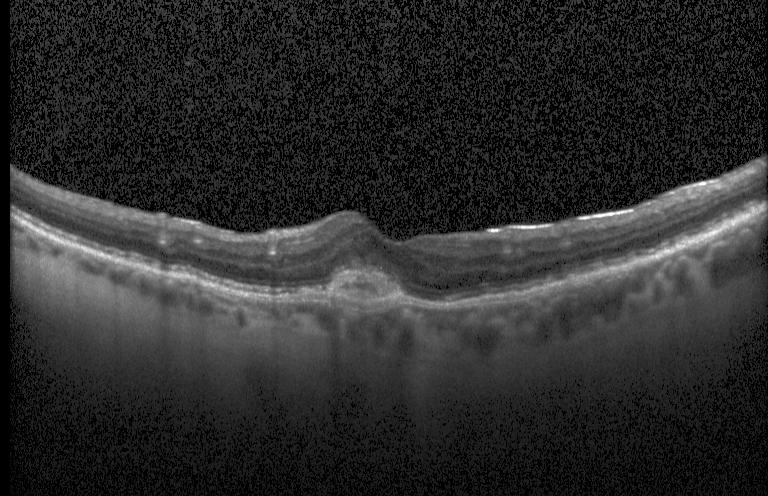 Spectral-domain OCT, macular scan, retinal OCT cross-section, acquired on a Heidelberg Spectralis — Macular OCT: choroidal neovascularization (CNV).